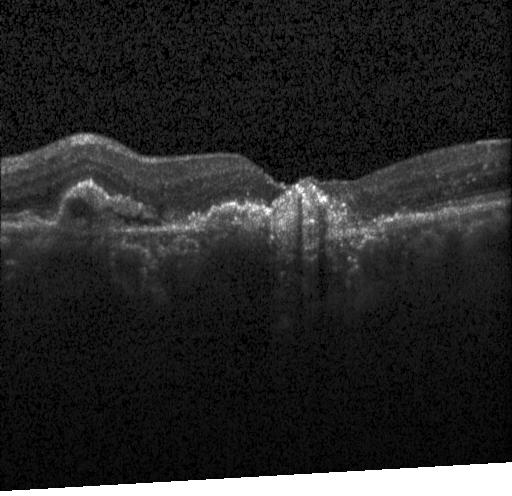 Retinal OCT cross-section showing a choroidal neovascular membrane.